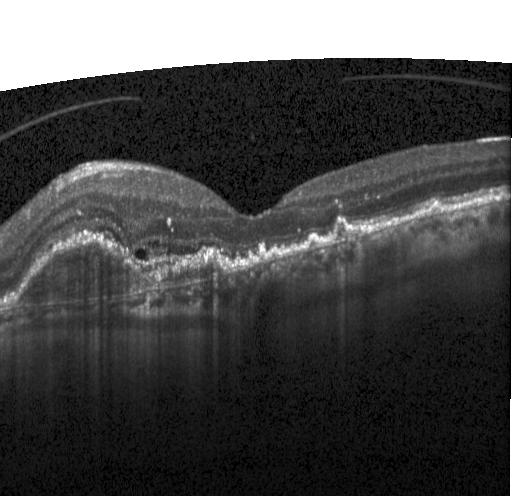
OCT line scan
Impression: CNV.